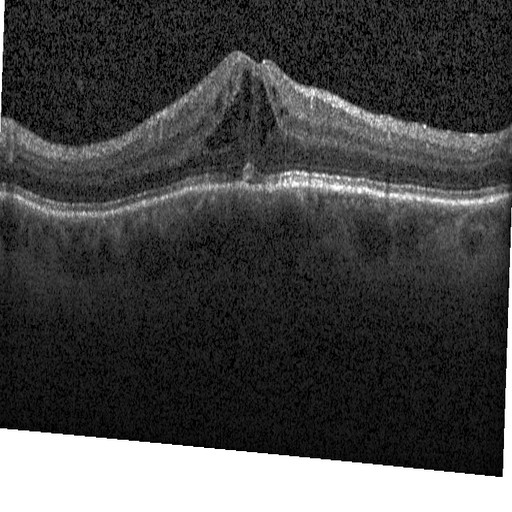 Retinal OCT cross-section.
Impression: DME.